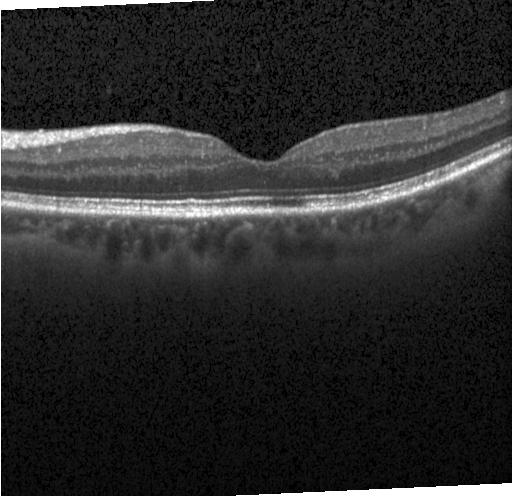
Spectral-domain optical coherence tomography. Optical coherence tomography scan.
This B-scan demonstrates no choroidal neovascularization, no diabetic macular edema, and no drusen.